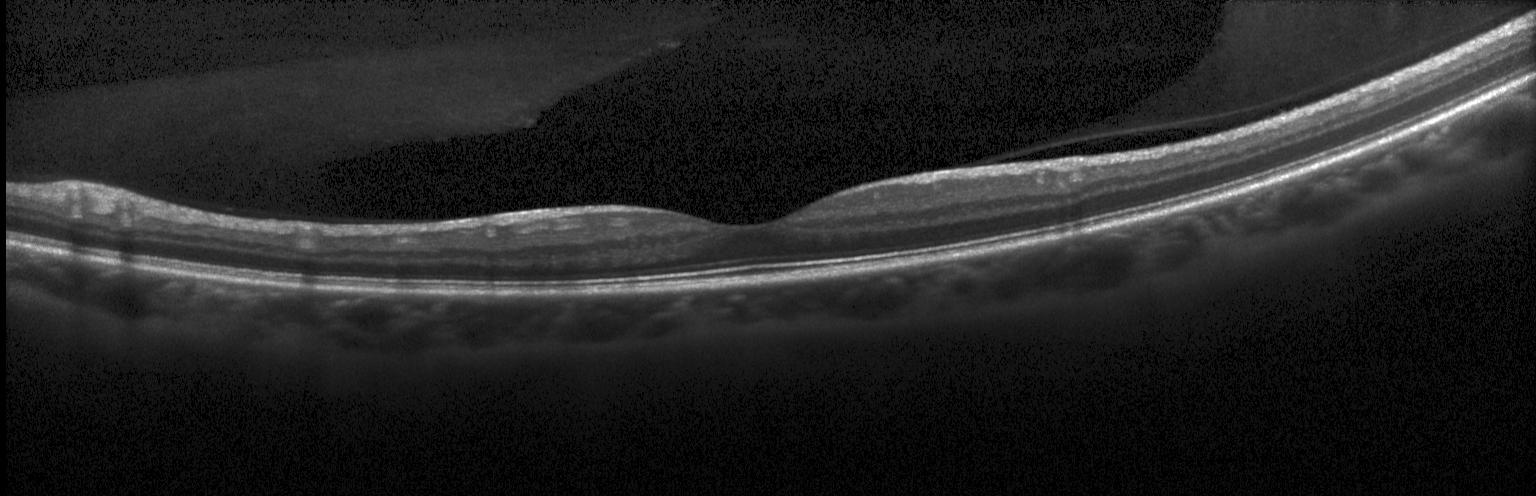 OCT line scan.
Impression: no evidence of choroidal neovascularization, diabetic macular edema, or drusen.